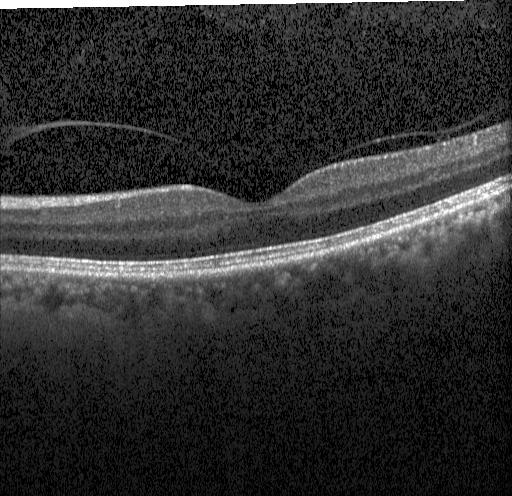 OCT B-scan. Instrument: Heidelberg Spectralis. Horizontal scan through the fovea. Spectral-domain optical coherence tomography — Diagnosis: no CNV, no DME, and no drusen.